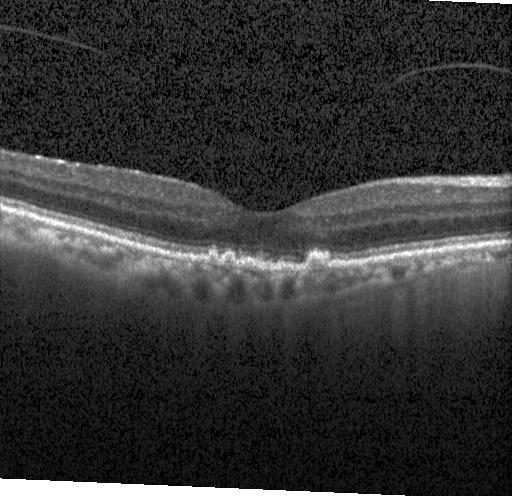
Fovea-centered. SD-OCT. Optical coherence tomography scan.
Diagnosis: sub-RPE drusenoid deposits.